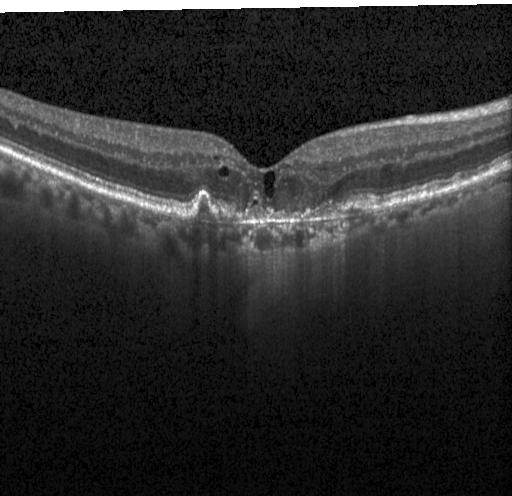

Diagnosis: choroidal neovascularization.